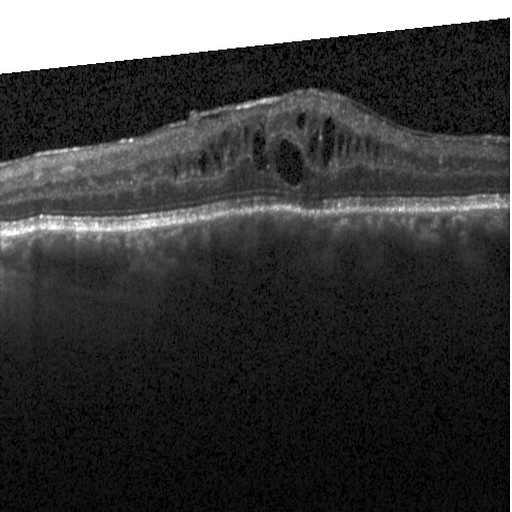 Diabetic macular edema (DME).